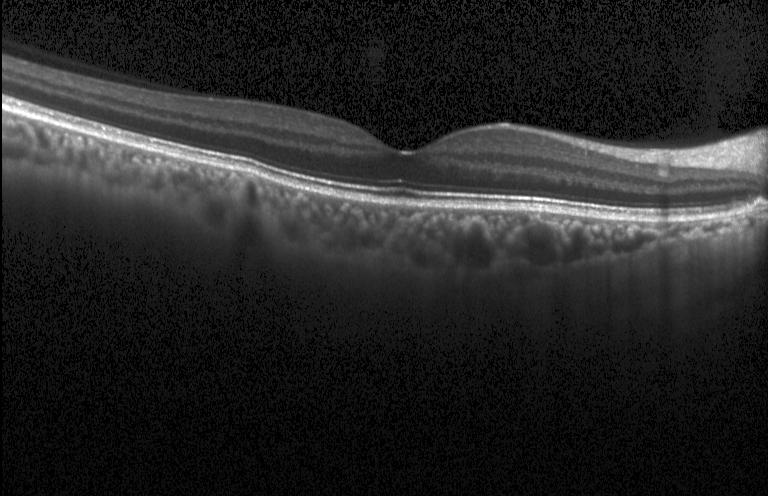 Retinal OCT B-scan, SD-OCT — OCT finding: no evidence of choroidal neovascularization, diabetic macular edema, or drusen.